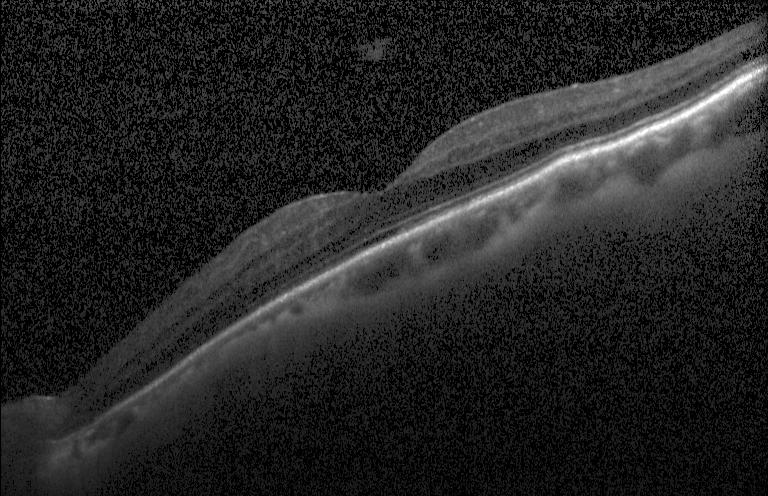 OCT line scan — Diagnosis: neither choroidal neovascularization, diabetic macular edema, nor drusen.